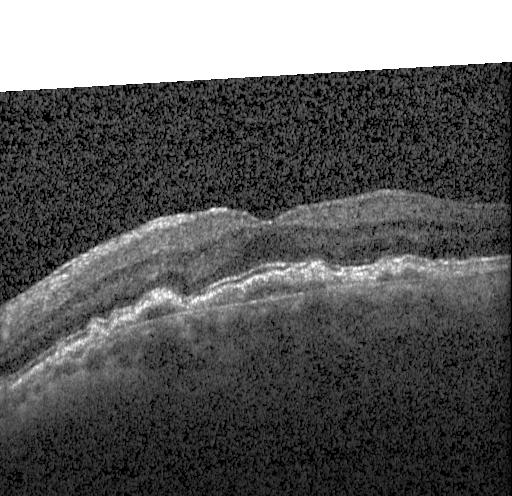

Dx: choroidal neovascularization.